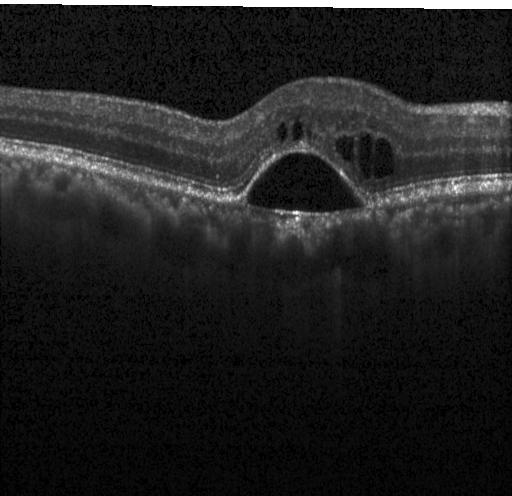

OCT line scan. Centered on the fovea — This B-scan demonstrates choroidal neovascularization.